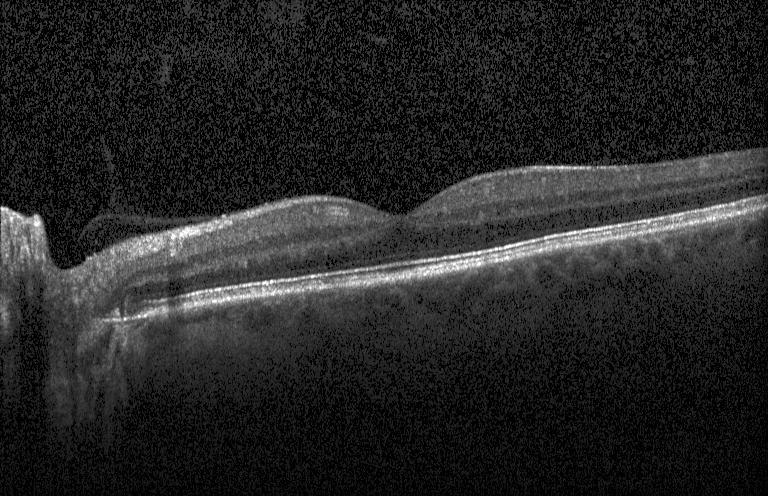

Dx: no CNV, no DME, and no drusen.